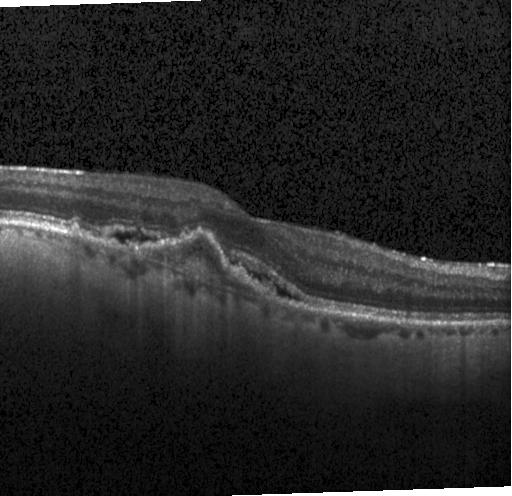
Dx: choroidal neovascularization (CNV).